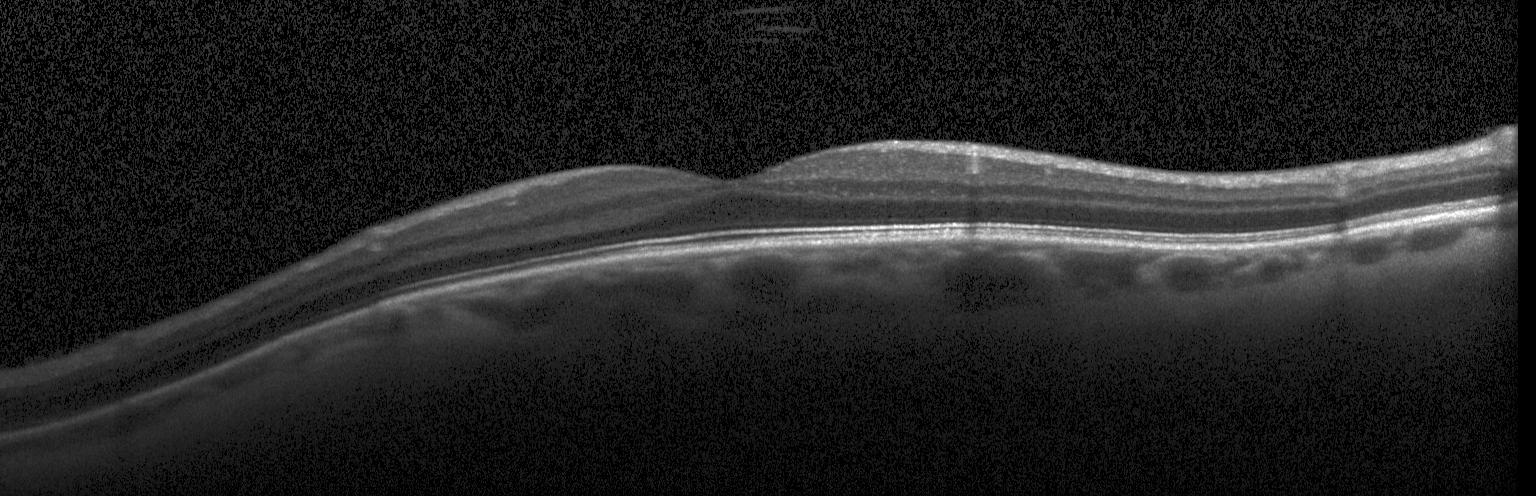 Macular OCT: neither CNV, DME, nor drusen.